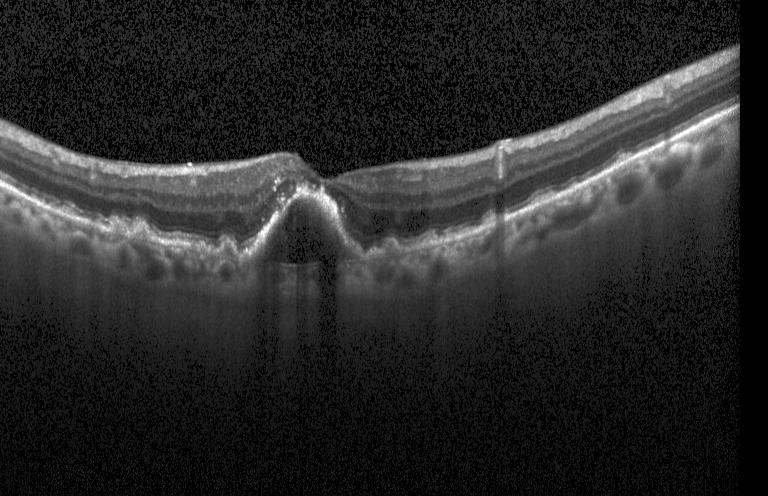 Optical coherence tomography B-scan; horizontal scan through the fovea; Heidelberg Spectralis; spectral-domain OCT. Finding: a choroidal neovascular membrane.